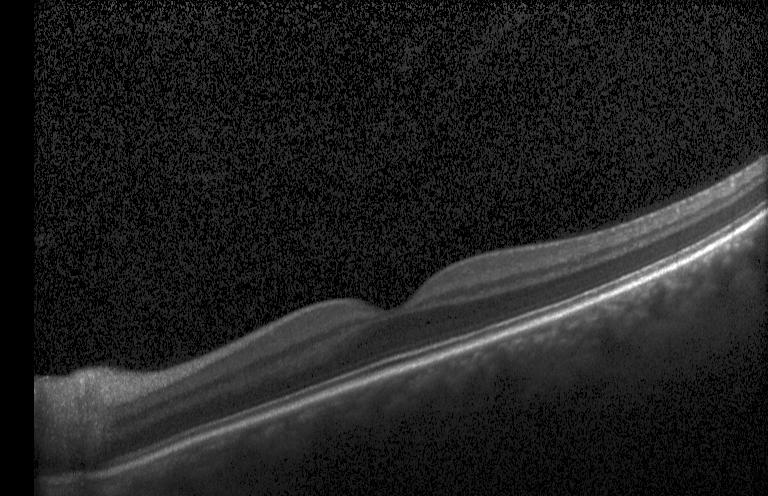 Macular scan. Optical coherence tomography B-scan. Heidelberg Spectralis OCT system.
The scan shows no choroidal neovascularization, no diabetic macular edema, and no drusen.